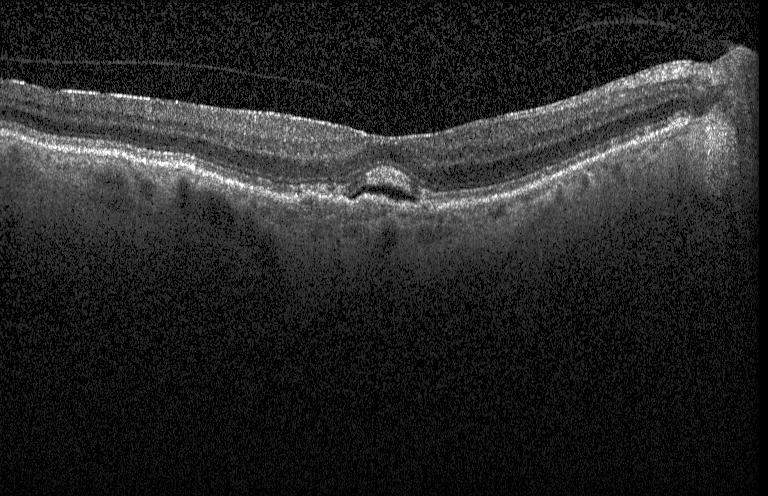 OCT B-scan; Heidelberg Spectralis; spectral-domain optical coherence tomography — Assessment: CNV.